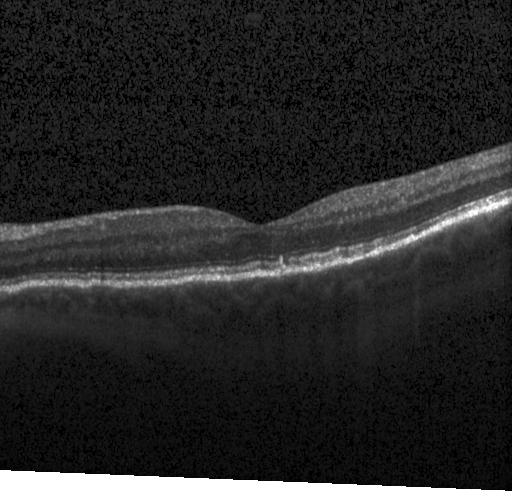
Optical coherence tomography scan.
Impression: multiple drusen.